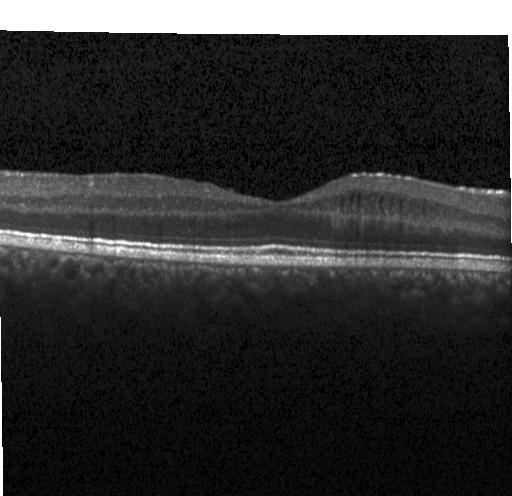
Spectral-domain optical coherence tomography; OCT B-scan; acquired on a Heidelberg Spectralis
The scan shows DME.